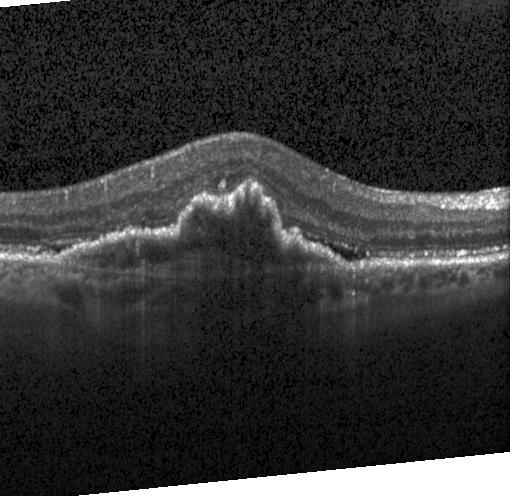
Fovea-centered · Heidelberg Spectralis · spectral-domain optical coherence tomography · optical coherence tomography B-scan — Dx: a choroidal neovascular membrane.